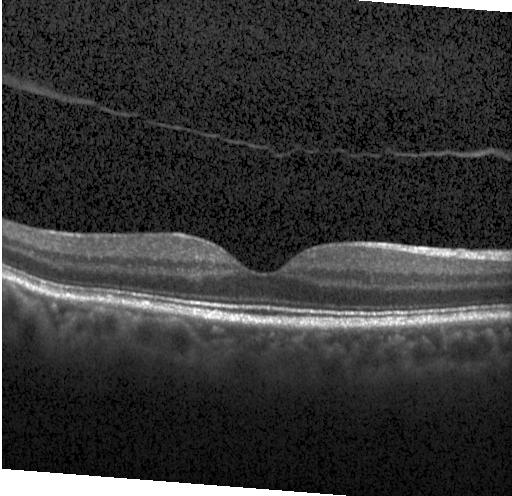
Optical coherence tomography scan.
Assessment: neither choroidal neovascularization, diabetic macular edema, nor drusen.